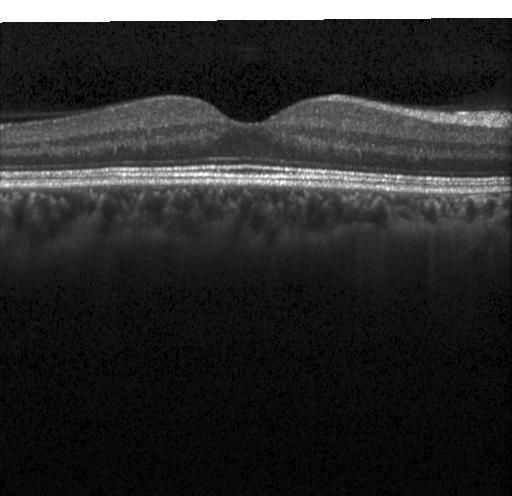 Macular OCT: no CNV, DME, or drusen.